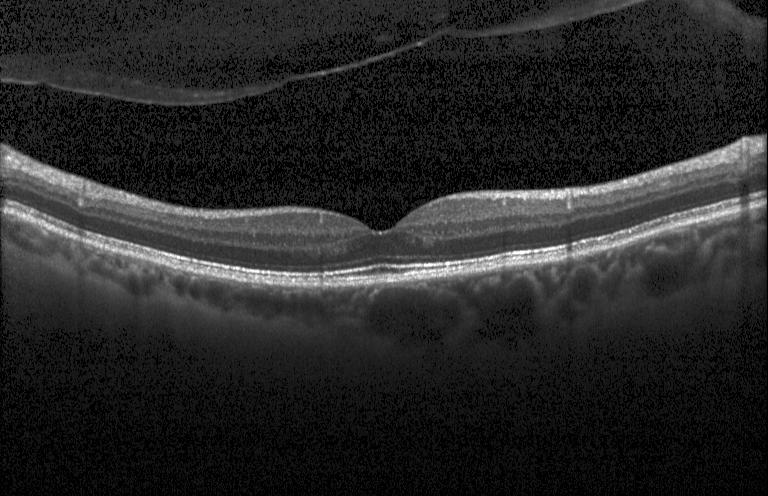
The scan shows neither choroidal neovascularization, diabetic macular edema, nor drusen.